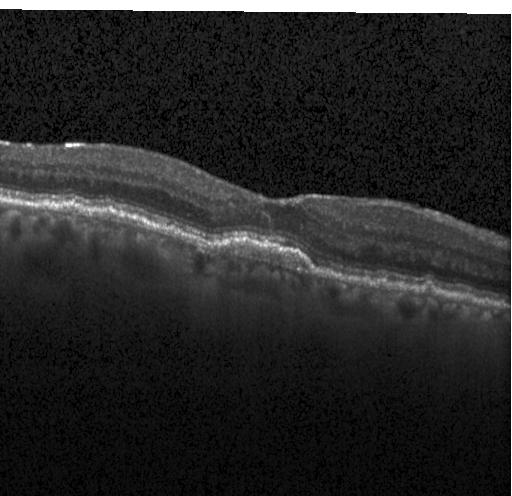 Instrument: Heidelberg Spectralis. Retinal OCT cross-section
CNV.